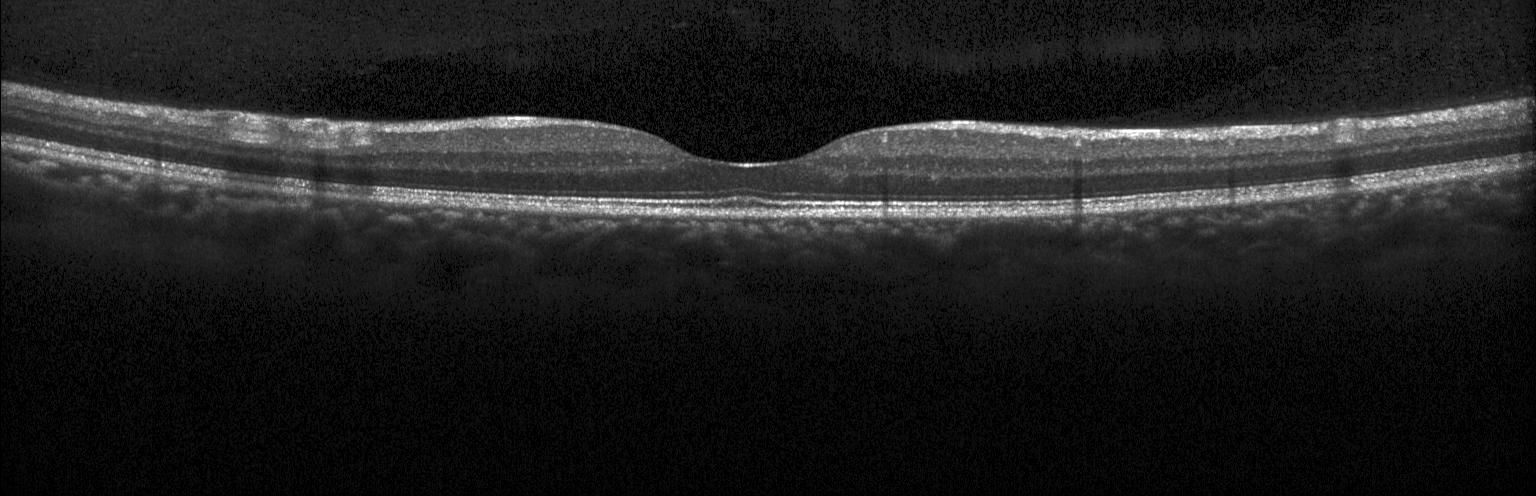
Dx: no CNV, DME, or drusen.